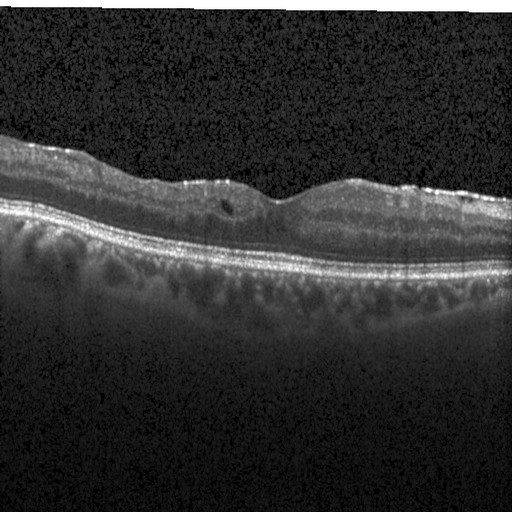
OCT B-scan — Diagnosis: DME.